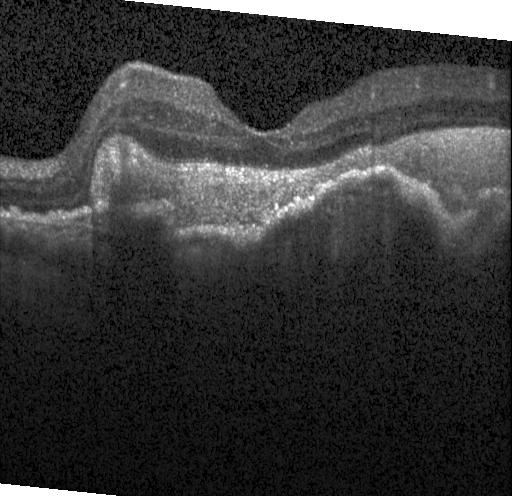

Optical coherence tomography scan; Heidelberg Spectralis OCT system; through the macula. The scan shows choroidal neovascularization.